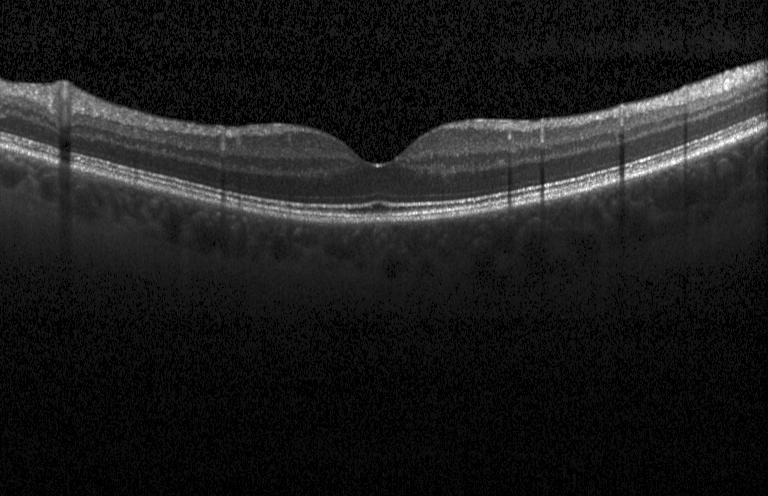 OCT B-scan — Impression: no choroidal neovascularization, diabetic macular edema, or drusen.